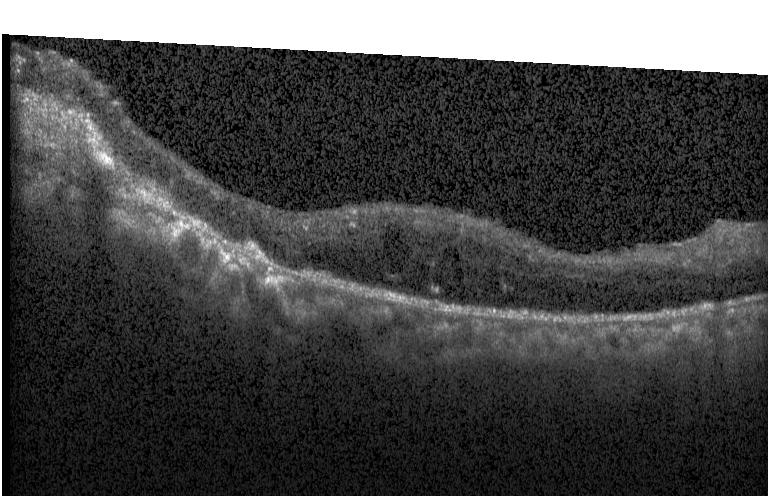

Optical coherence tomography scan, Heidelberg Spectralis OCT system
Finding: diabetic macular edema (DME).